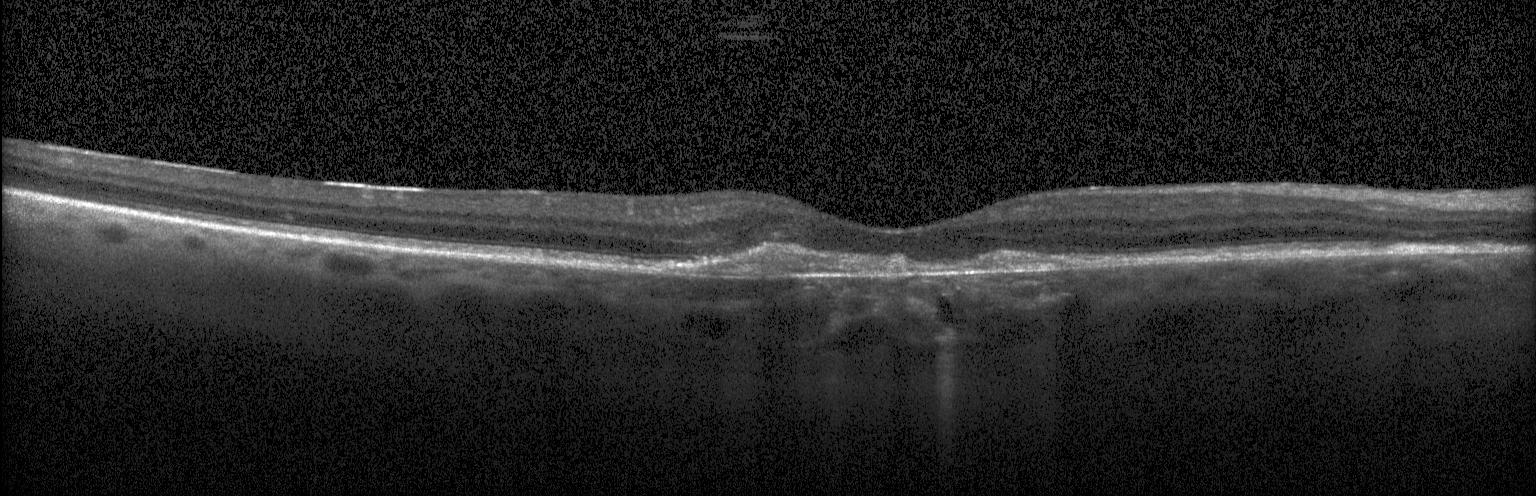

Impression: choroidal neovascularization.